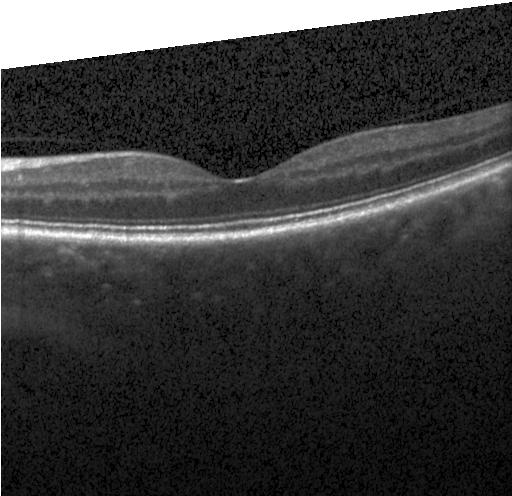 Macular OCT: no choroidal neovascularization, no diabetic macular edema, and no drusen.